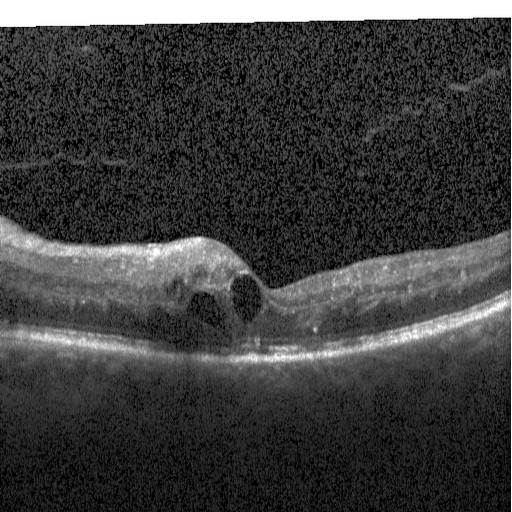 Optical coherence tomography scan
Impression: diabetic macular edema (DME).